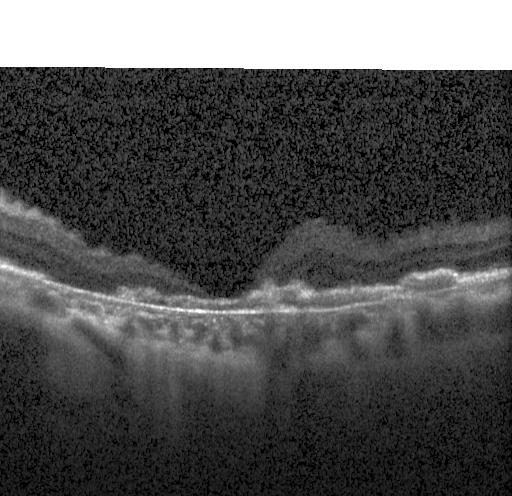
Heidelberg Spectralis · fovea-centered · OCT B-scan. Finding: choroidal neovascularization.